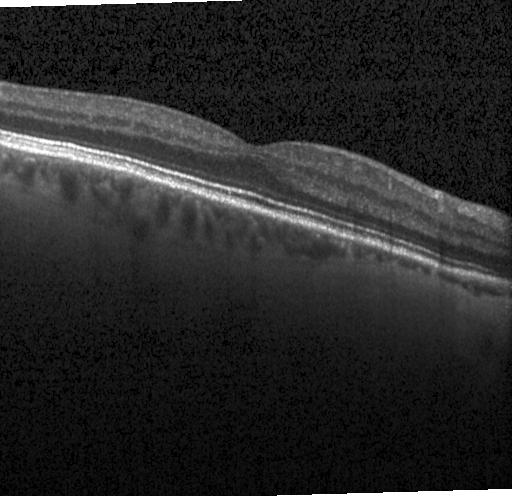

Instrument: Heidelberg Spectralis, through the macula, spectral-domain OCT, retinal OCT cross-section.
Macular OCT: no choroidal neovascularization, diabetic macular edema, or drusen.